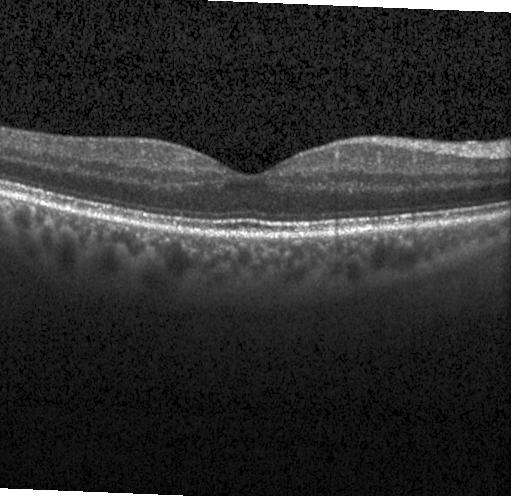

This B-scan demonstrates neither choroidal neovascularization, diabetic macular edema, nor drusen.